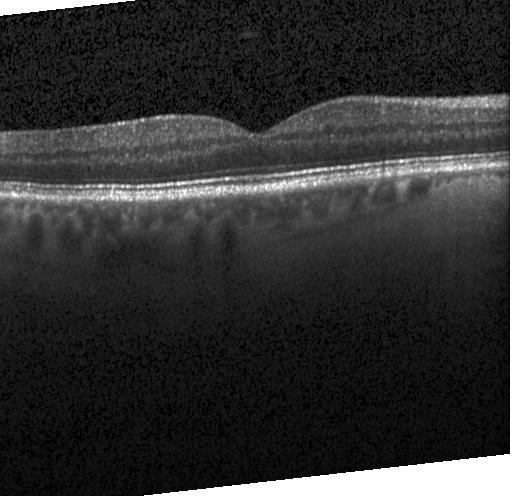 SD-OCT. Macular scan. Acquired on a Heidelberg Spectralis. Retinal OCT cross-section. Impression: neither choroidal neovascularization, diabetic macular edema, nor drusen.